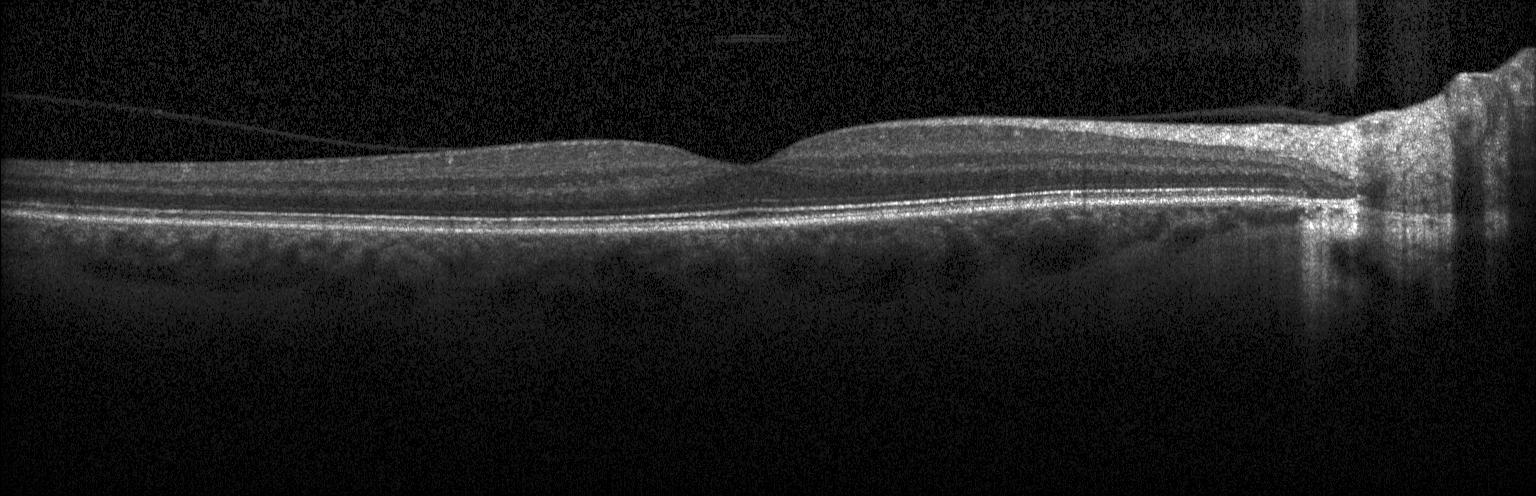

OCT line scan.
Dx: no choroidal neovascularization, no diabetic macular edema, and no drusen.